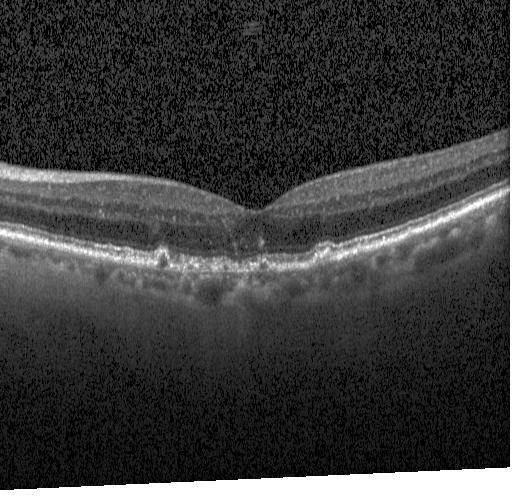
Acquired on a Heidelberg Spectralis · optical coherence tomography scan
A choroidal neovascular membrane.